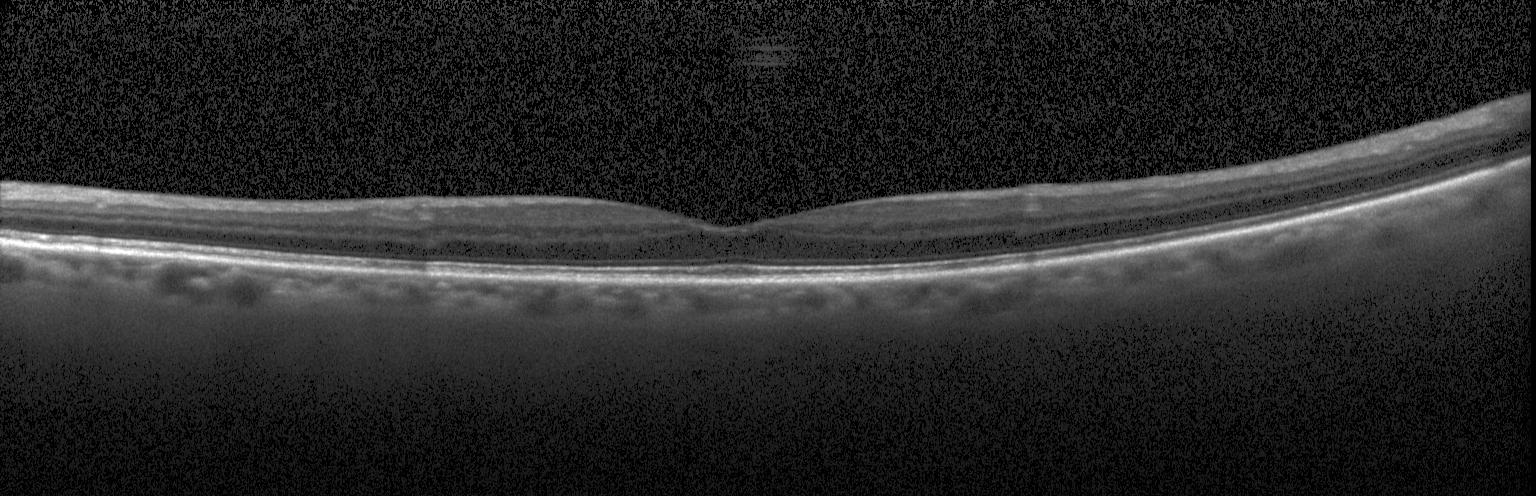
Fovea-centered. OCT B-scan. Acquired on a Heidelberg Spectralis. Impression: no choroidal neovascularization, no diabetic macular edema, and no drusen.